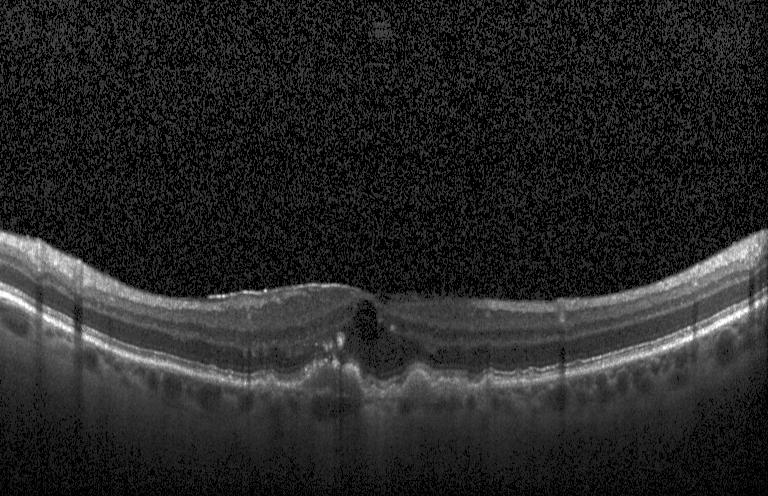 Spectral-domain optical coherence tomography; acquired on a Heidelberg Spectralis; optical coherence tomography B-scan; horizontal scan through the fovea — Assessment: a choroidal neovascular membrane.